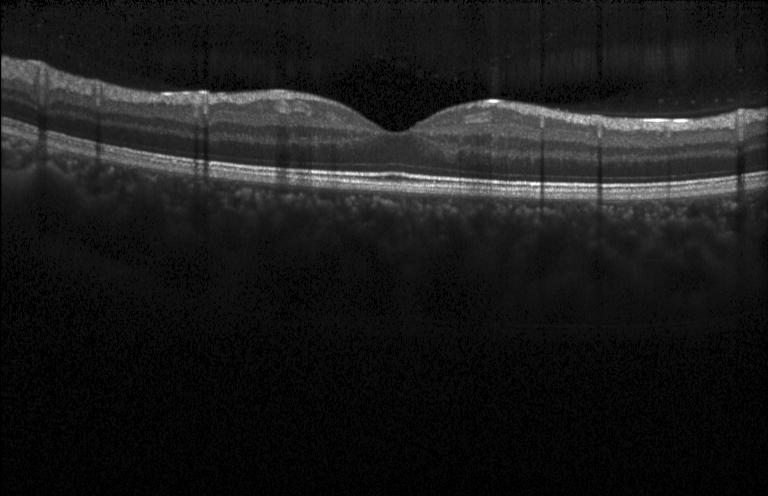
OCT scan showing no choroidal neovascularization, diabetic macular edema, or drusen.